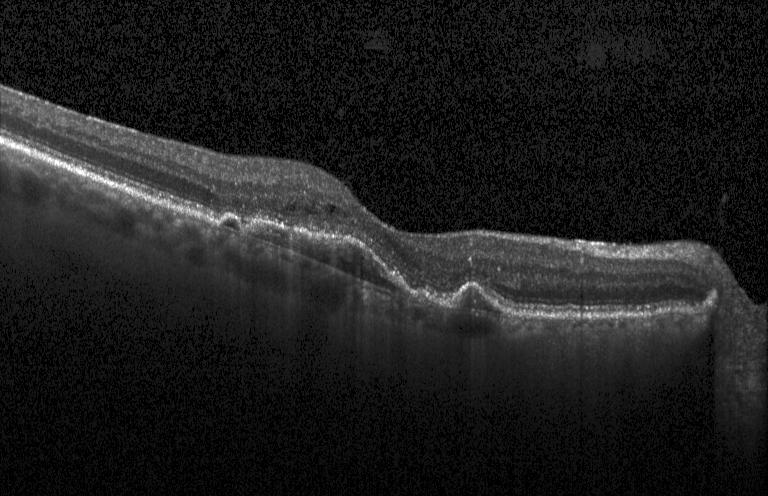

Retinal OCT B-scan. Macular OCT: CNV.